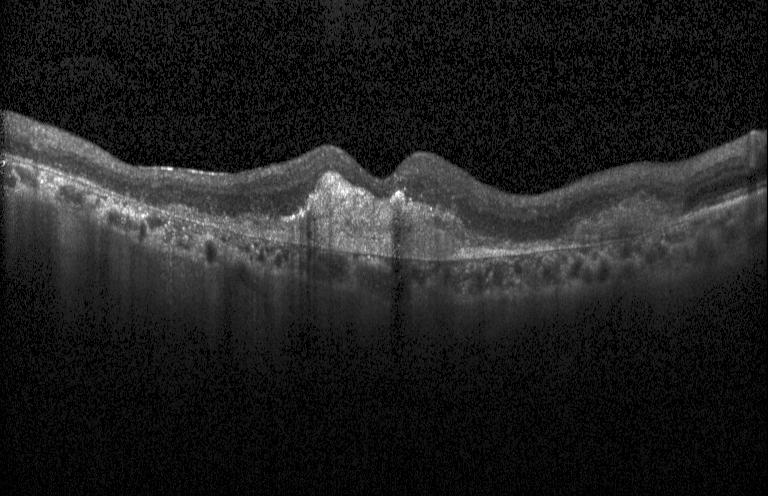
OCT scan showing choroidal neovascularization.